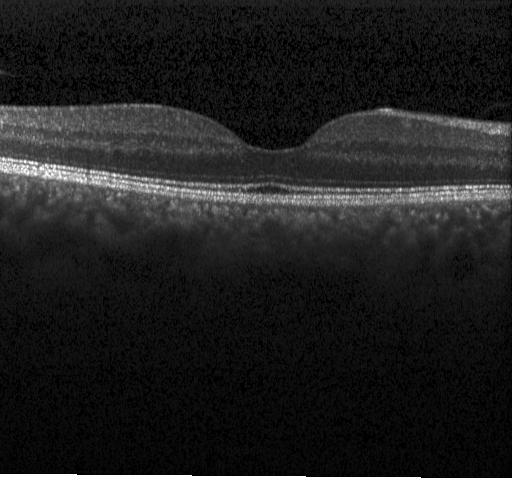
Retinal OCT B-scan, centered on the fovea, SD-OCT, Heidelberg Spectralis OCT system.
OCT finding: no CNV, no DME, and no drusen.